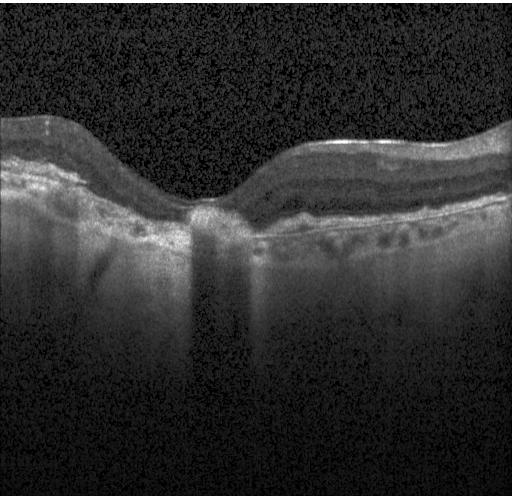

OCT finding: choroidal neovascularization (CNV).